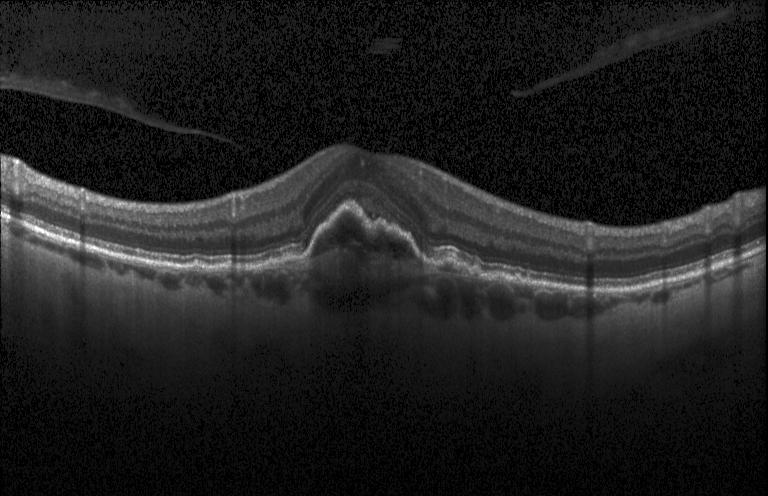
Through the macula. SD-OCT. Acquired on a Heidelberg Spectralis. OCT B-scan
Impression: choroidal neovascularization (CNV).